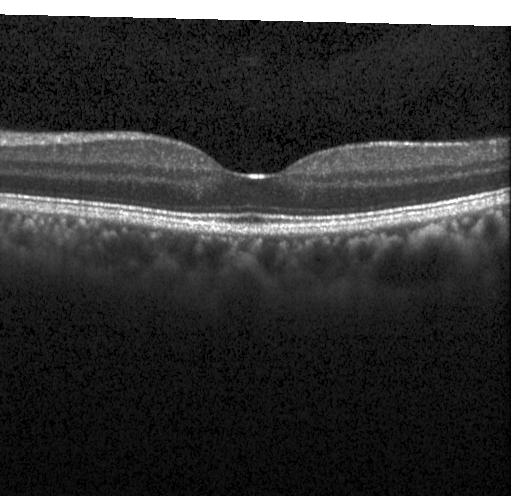
No CNV, no DME, and no drusen.